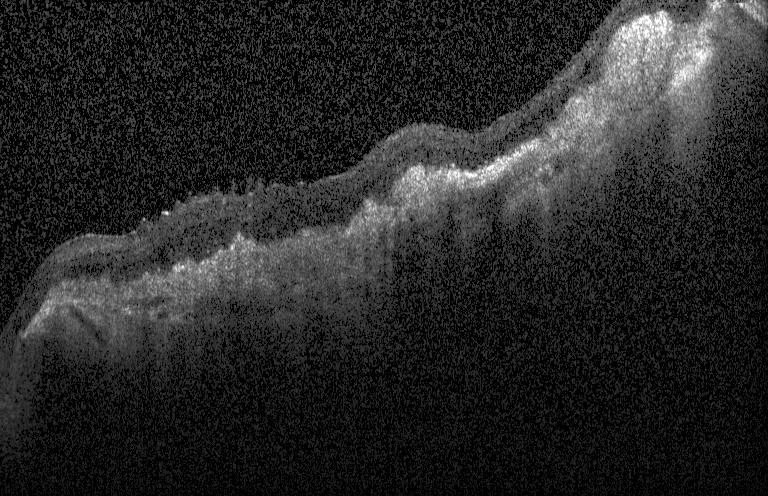
Macular OCT: a choroidal neovascular membrane.